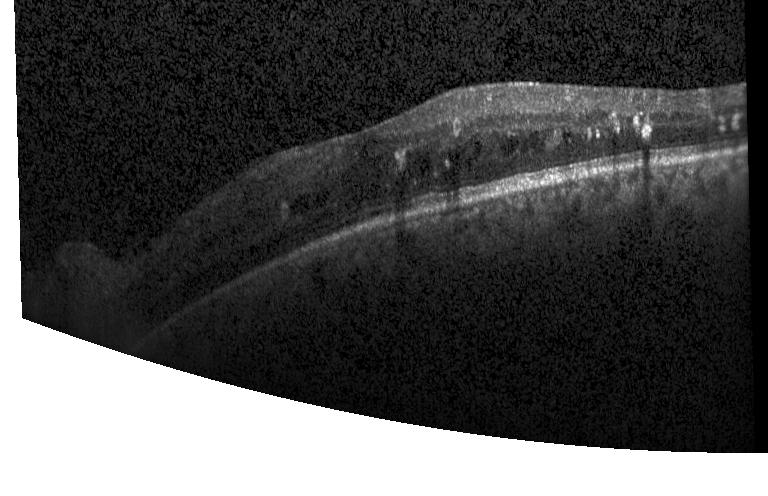 Impression: diabetic macular edema.